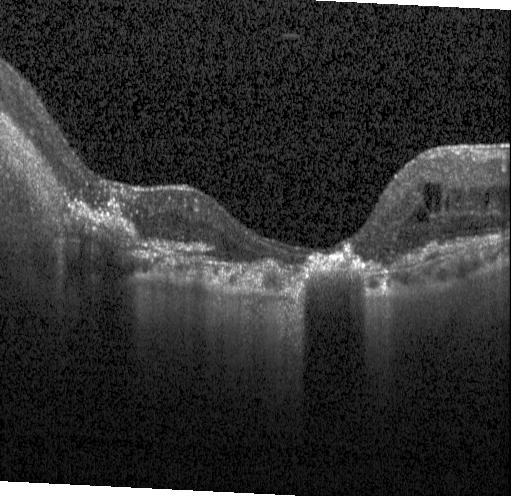

OCT finding: choroidal neovascularization (CNV).